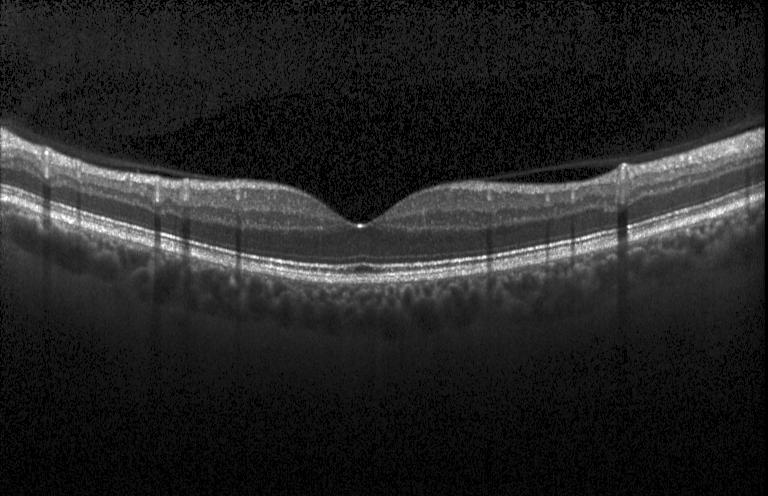
OCT B-scan · horizontal scan through the fovea
Assessment: no choroidal neovascularization, diabetic macular edema, or drusen.